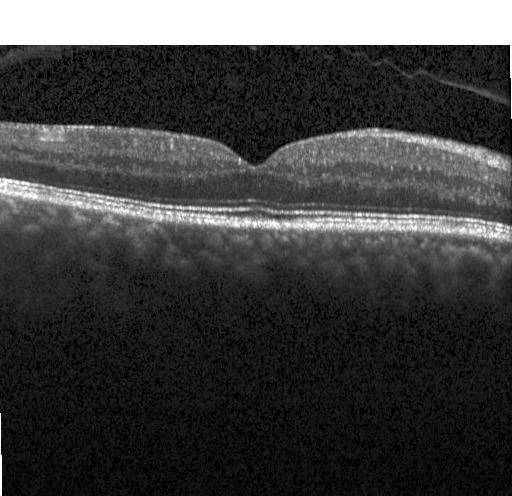 Retinal OCT B-scan · Heidelberg Spectralis · through the macula · SD-OCT
Diagnosis: no choroidal neovascularization, diabetic macular edema, or drusen.